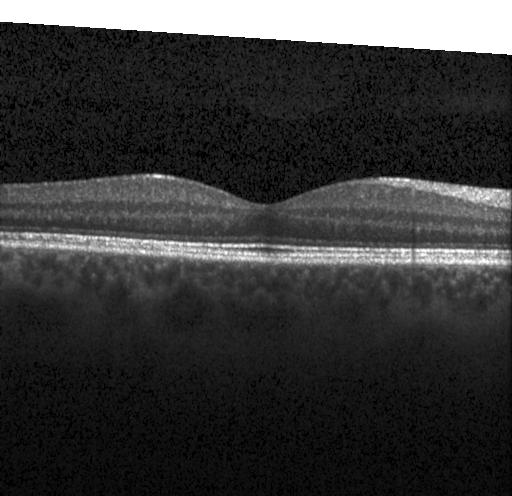 Heidelberg Spectralis OCT system, spectral-domain OCT, optical coherence tomography scan. Finding: no choroidal neovascularization, diabetic macular edema, or drusen.